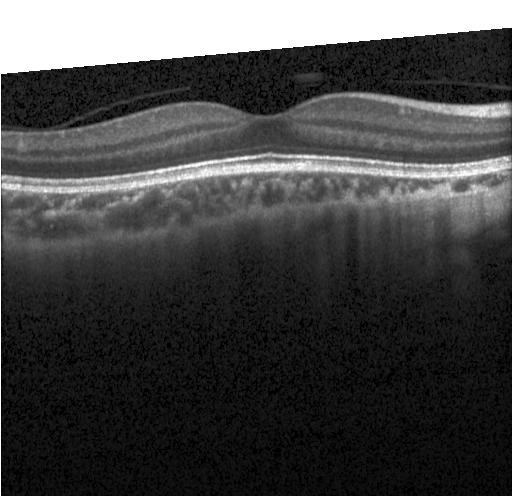
Retinal OCT B-scan
Dx: no CNV, DME, or drusen.